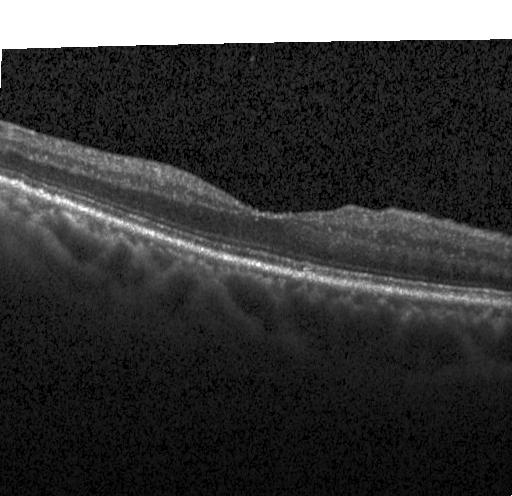 Diagnosis: neither choroidal neovascularization, diabetic macular edema, nor drusen.